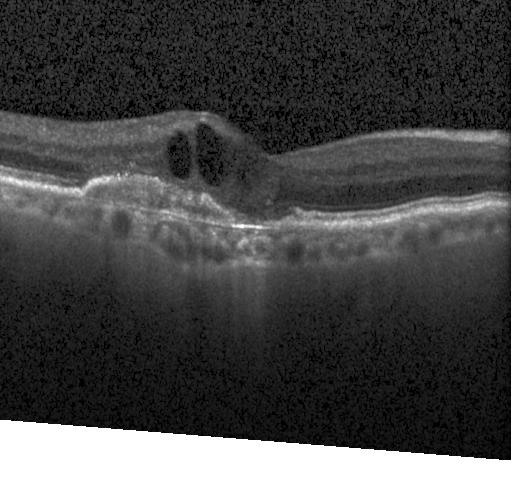 Spectral-domain OCT B-scan: a choroidal neovascular membrane.